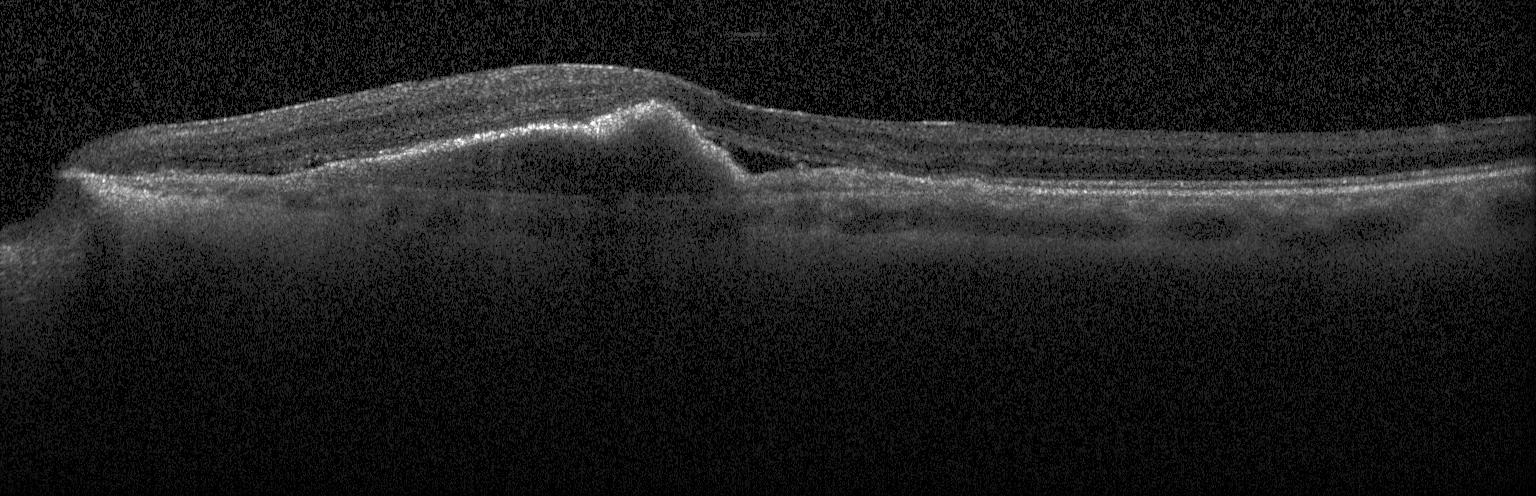
OCT scan showing a choroidal neovascular membrane.